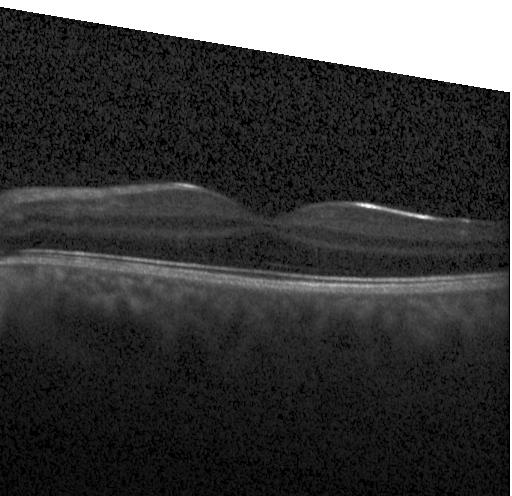 Macular OCT: no choroidal neovascularization, no diabetic macular edema, and no drusen.